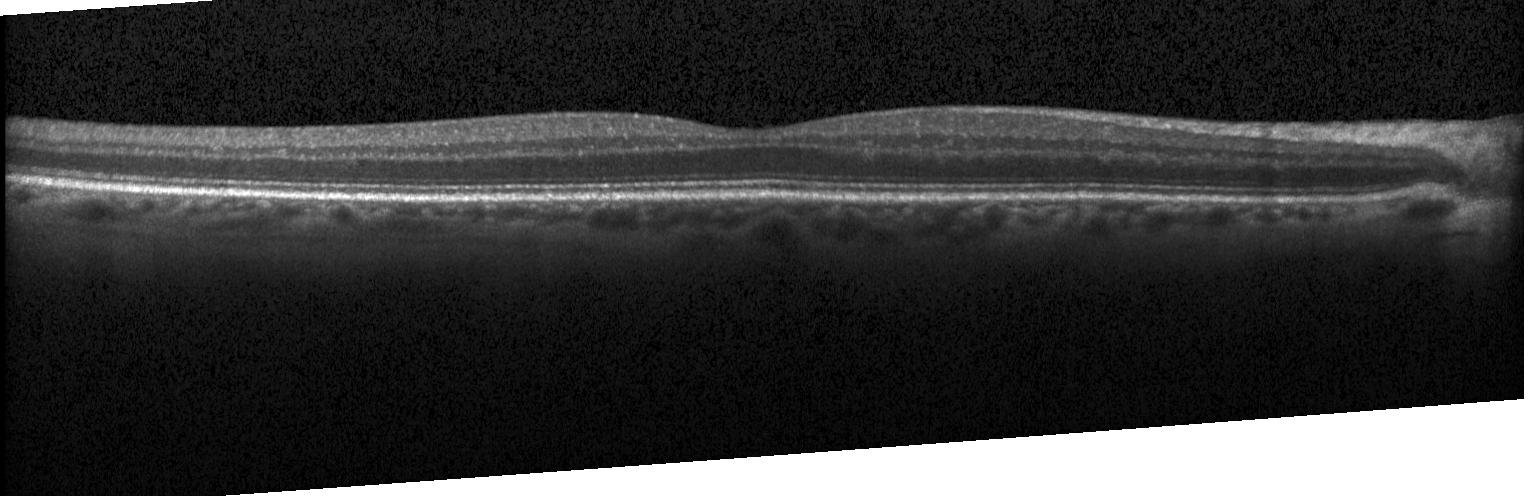 Macular scan, optical coherence tomography B-scan — OCT finding: no choroidal neovascularization, no diabetic macular edema, and no drusen.